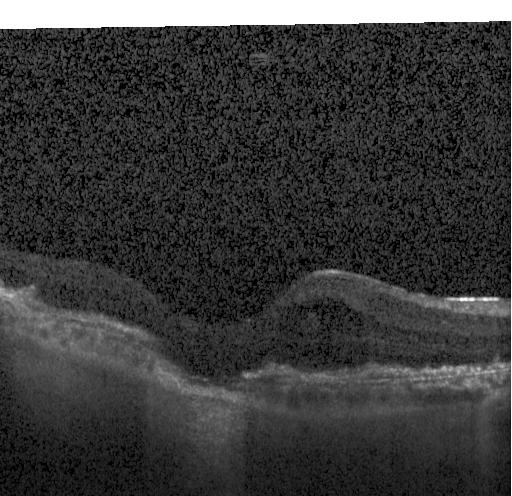
The scan shows CNV.